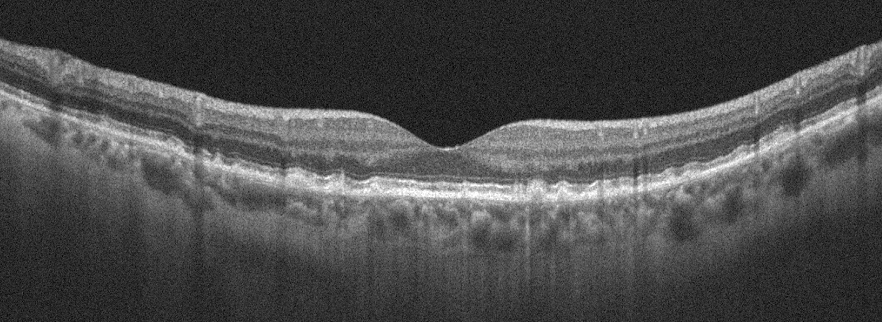 OD; retinal OCT cross-section
Age-related macular degeneration.